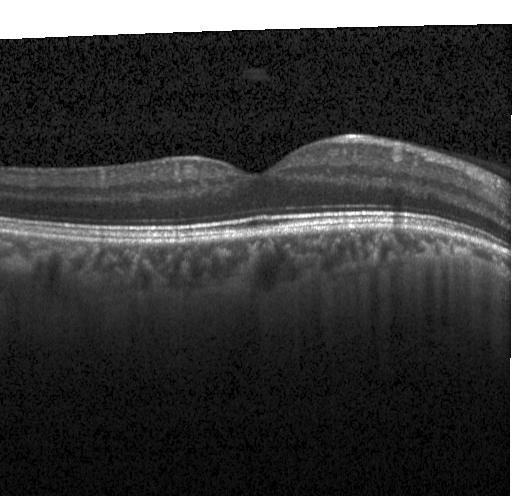

Spectral-domain OCT. Acquired on a Heidelberg Spectralis. Centered on the fovea. Optical coherence tomography B-scan — Finding: no choroidal neovascularization, diabetic macular edema, or drusen.